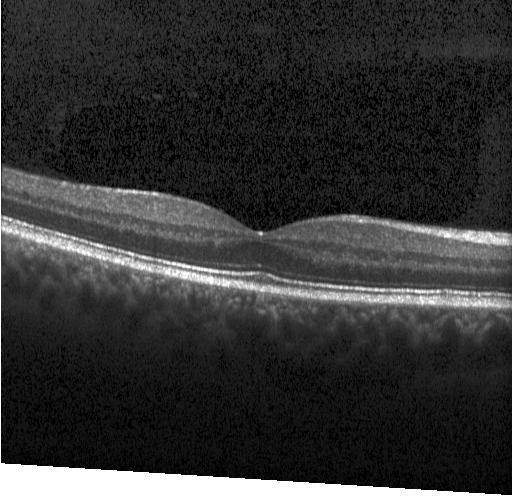

Spectral-domain OCT · macular scan · acquired on a Heidelberg Spectralis · OCT line scan. Impression: no evidence of choroidal neovascularization, diabetic macular edema, or drusen.